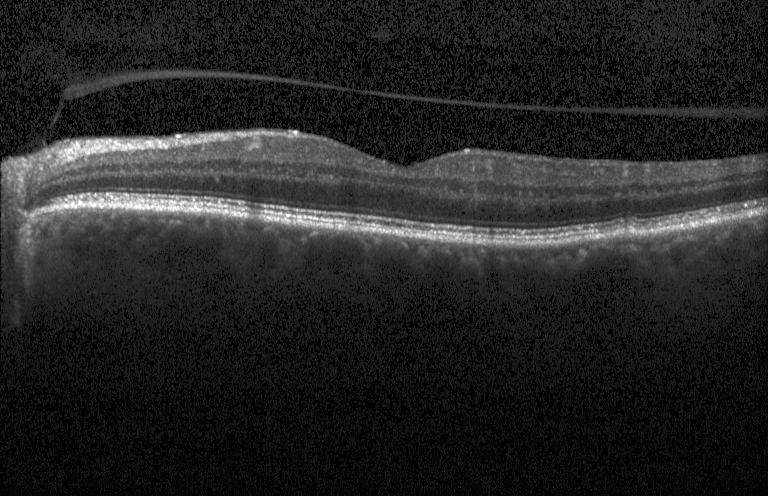 Instrument: Heidelberg Spectralis. Retinal OCT cross-section. Centered on the fovea. SD-OCT. Assessment: neither CNV, DME, nor drusen.